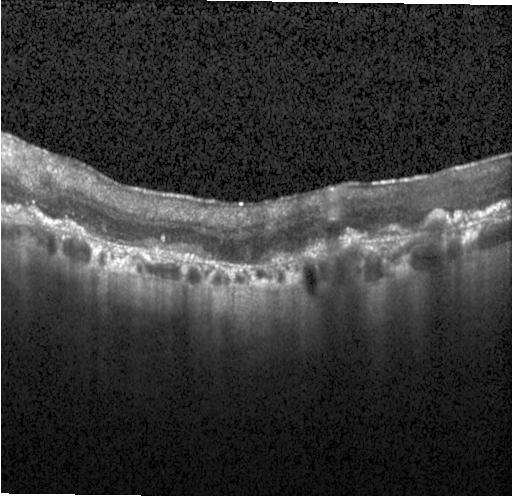 Fovea-centered · optical coherence tomography scan · acquired on a Heidelberg Spectralis.
The scan shows CNV.